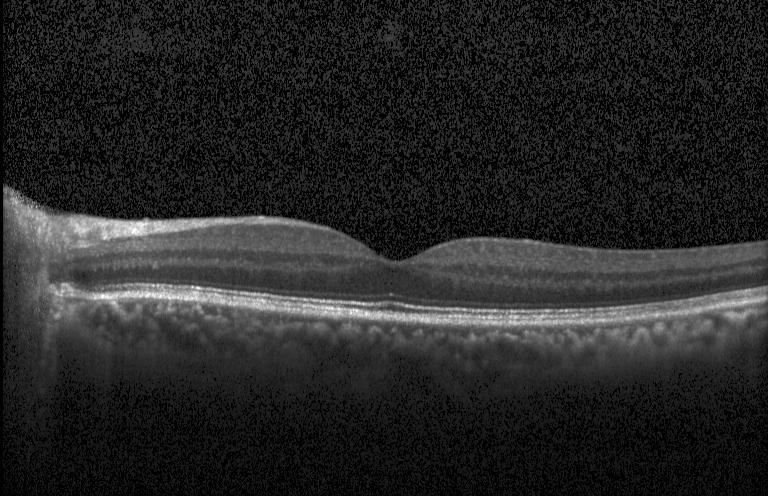

Diagnosis: no CNV, no DME, and no drusen.